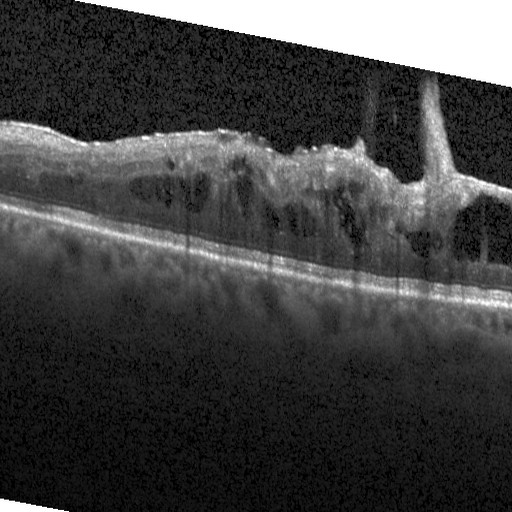 Spectral-domain optical coherence tomography. Through the macula. Optical coherence tomography B-scan. Heidelberg Spectralis OCT system.
Impression: DME.